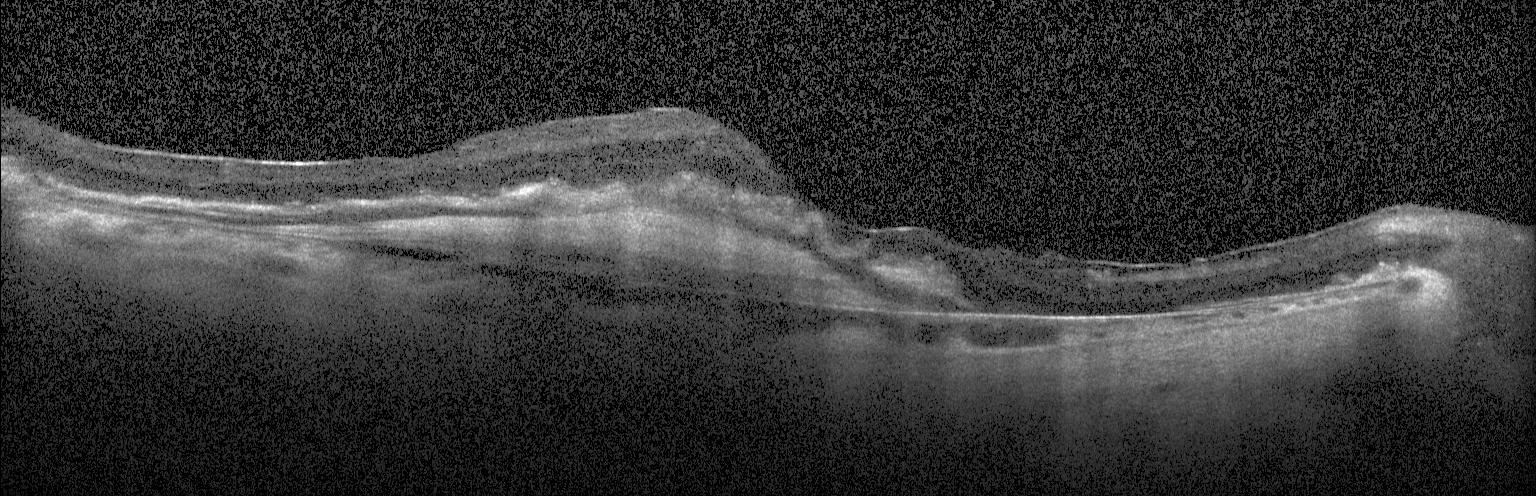

Instrument: Heidelberg Spectralis, optical coherence tomography B-scan, spectral-domain OCT
Diagnosis: choroidal neovascularization.